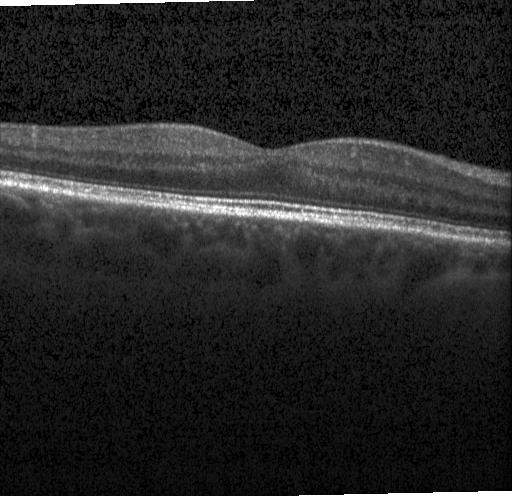 Retinal OCT B-scan; spectral-domain optical coherence tomography; Heidelberg Spectralis OCT system; fovea-centered
Dx: no choroidal neovascularization, no diabetic macular edema, and no drusen.